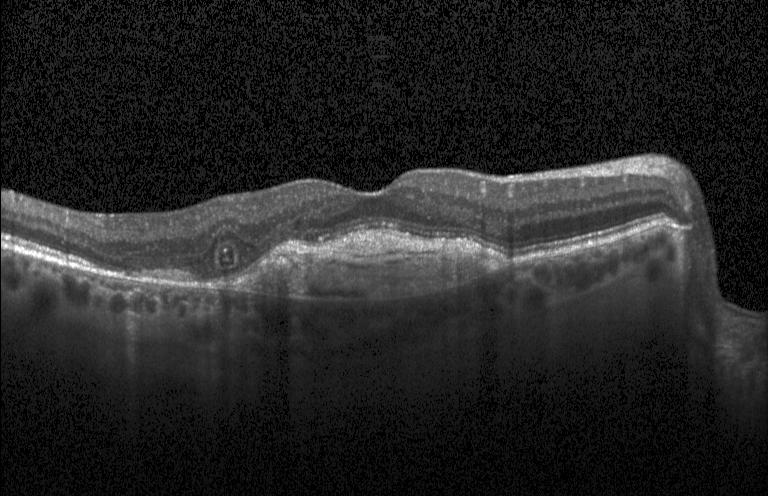

Impression: CNV.